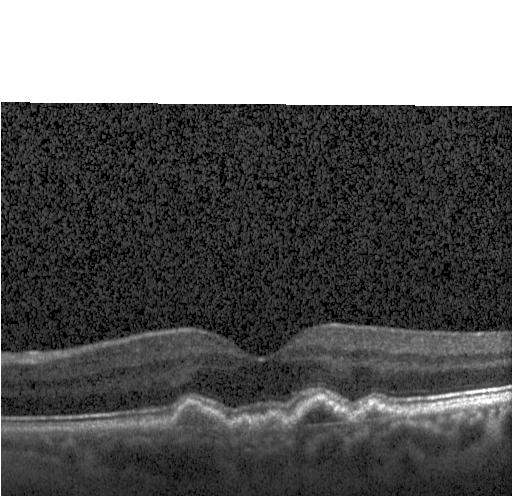
OCT B-scan.
This B-scan demonstrates sub-RPE drusenoid deposits.